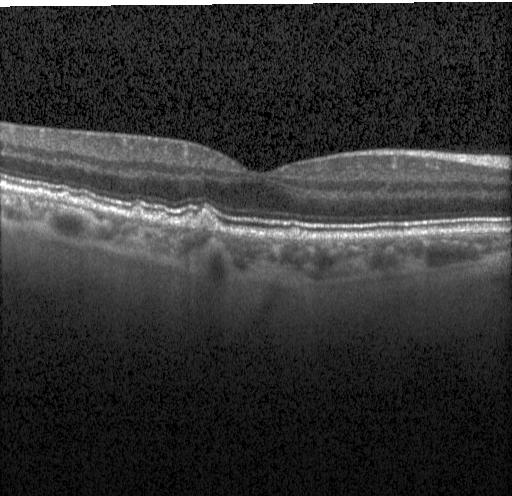 Retinal OCT cross-section, Heidelberg Spectralis OCT system, spectral-domain OCT, centered on the fovea — Diagnosis: sub-RPE drusenoid deposits.